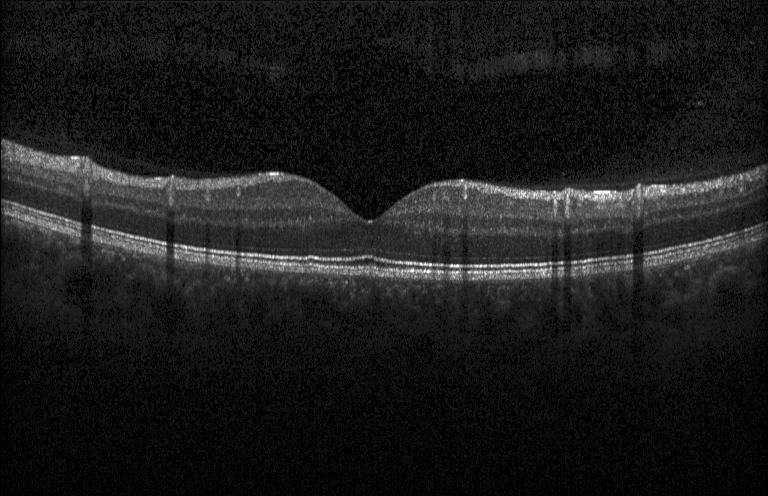
Macular OCT demonstrating no CNV, no DME, and no drusen.